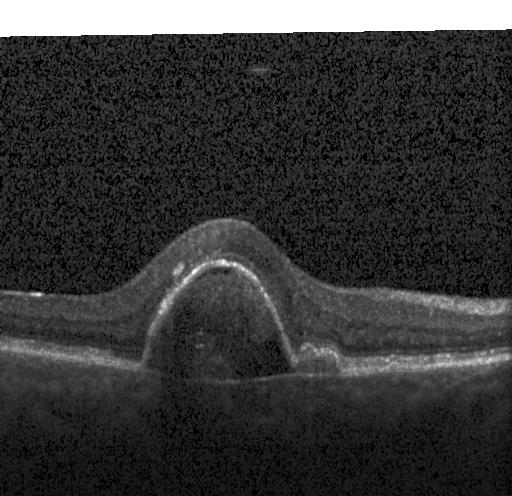

Heidelberg Spectralis. Spectral-domain optical coherence tomography. OCT B-scan. Through the macula. The scan shows a choroidal neovascular membrane.